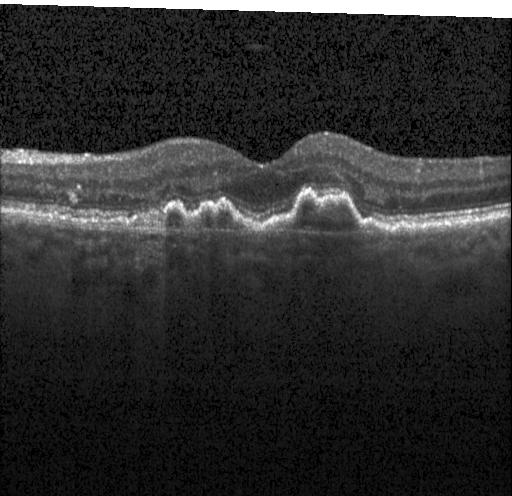

Dx: a choroidal neovascular membrane.